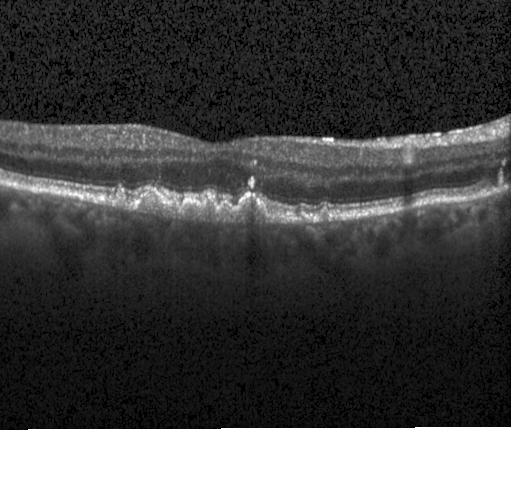
Heidelberg Spectralis OCT system · optical coherence tomography scan · centered on the fovea · SD-OCT — Finding: multiple drusen.